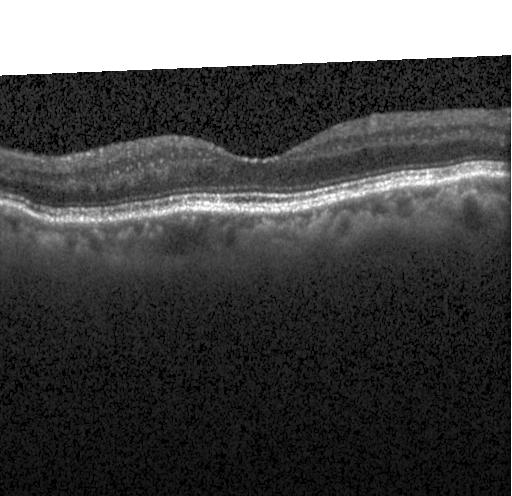
OCT line scan; horizontal scan through the fovea.
Impression: neither CNV, DME, nor drusen.